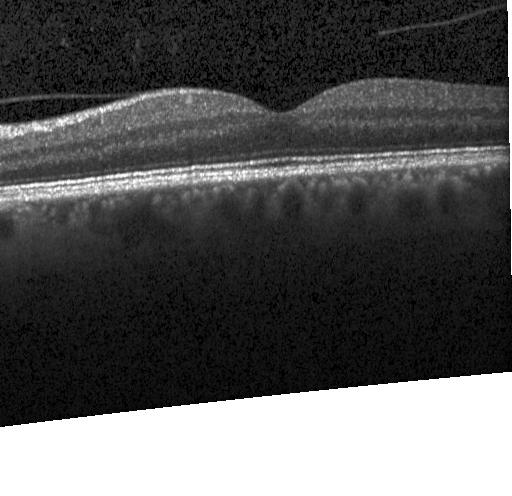
Horizontal scan through the fovea · spectral-domain optical coherence tomography · retinal OCT B-scan
Finding: neither CNV, DME, nor drusen.